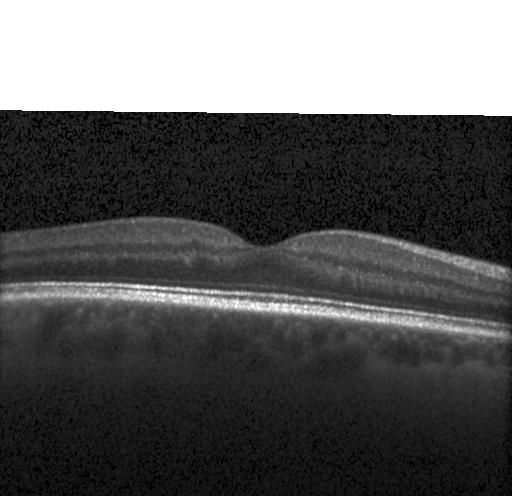
Spectral-domain optical coherence tomography, OCT B-scan, acquired on a Heidelberg Spectralis, fovea-centered. Macular OCT: neither choroidal neovascularization, diabetic macular edema, nor drusen.